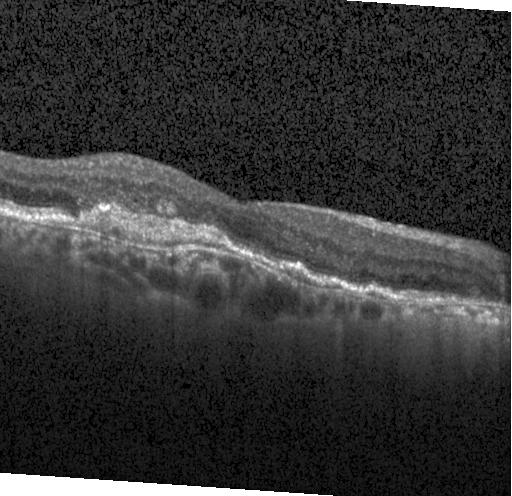
Spectral-domain OCT, optical coherence tomography B-scan, Heidelberg Spectralis, through the macula.
Diagnosis: choroidal neovascularization.